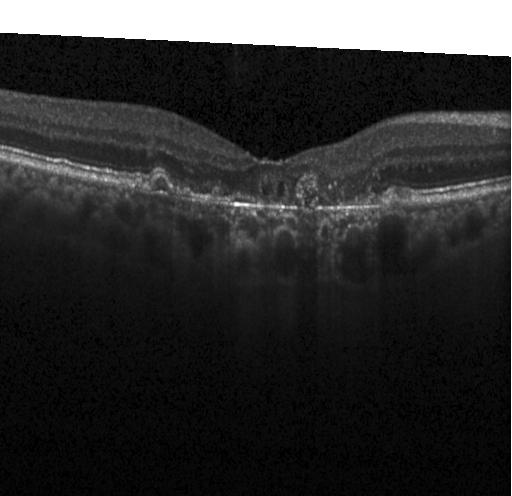

Spectral-domain optical coherence tomography · OCT line scan.
This B-scan demonstrates a choroidal neovascular membrane.